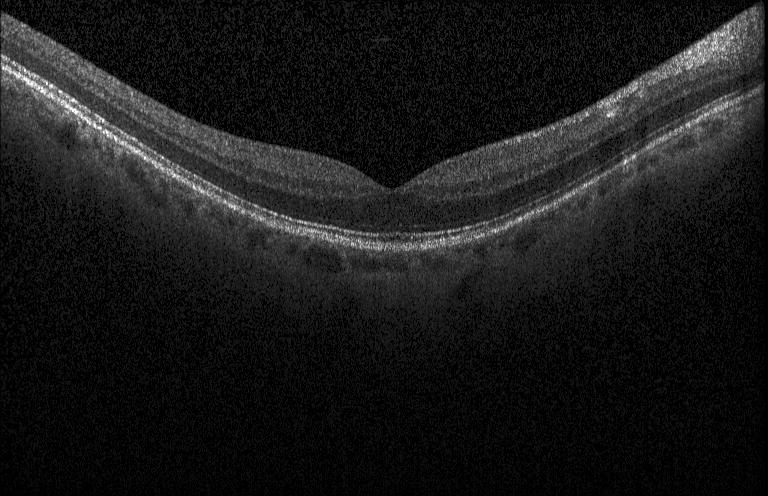
OCT scan showing neither CNV, DME, nor drusen.